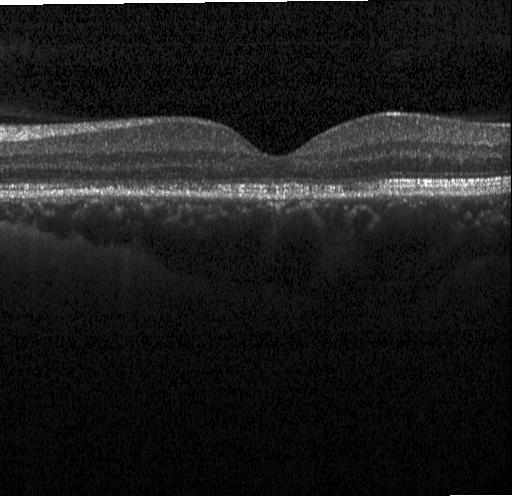
SD-OCT; retinal OCT cross-section. Impression: no choroidal neovascularization, no diabetic macular edema, and no drusen.